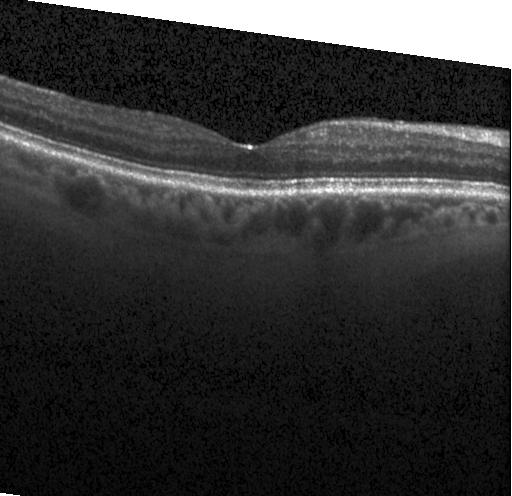
Macular scan · optical coherence tomography B-scan · instrument: Heidelberg Spectralis · spectral-domain OCT. No choroidal neovascularization, no diabetic macular edema, and no drusen.